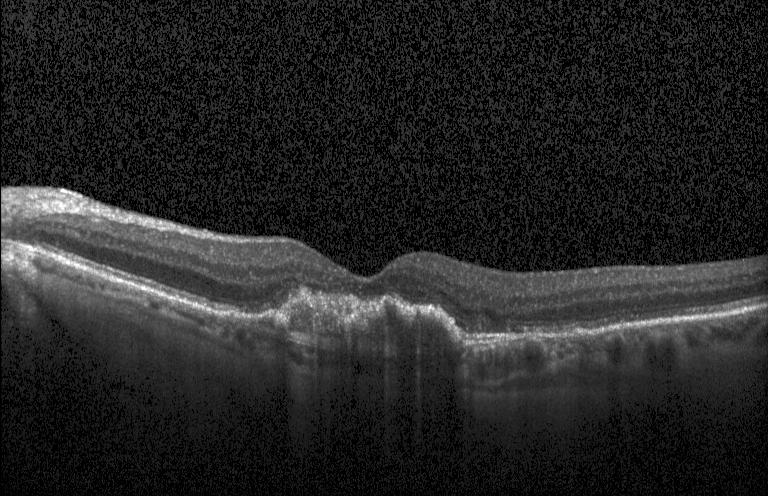
Retinal OCT cross-section — This B-scan demonstrates a choroidal neovascular membrane.